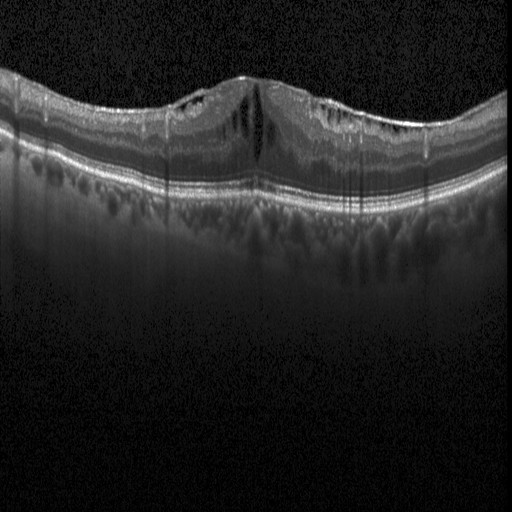
OCT B-scan; centered on the fovea; spectral-domain optical coherence tomography; Heidelberg Spectralis. This B-scan demonstrates DME.